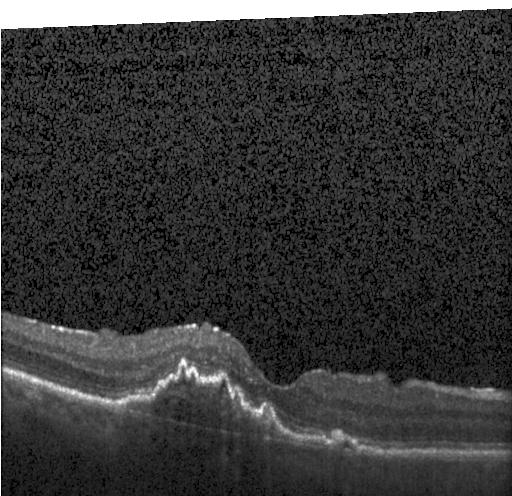

Optical coherence tomography B-scan · acquired on a Heidelberg Spectralis · through the macula · SD-OCT — Dx: a choroidal neovascular membrane.